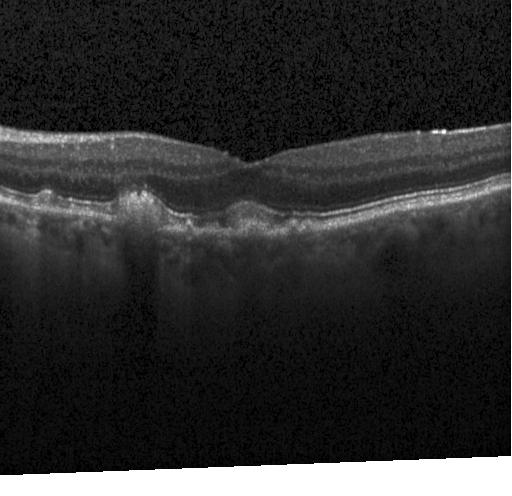
Optical coherence tomography scan. Heidelberg Spectralis. Horizontal scan through the fovea
Dx: a choroidal neovascular membrane.